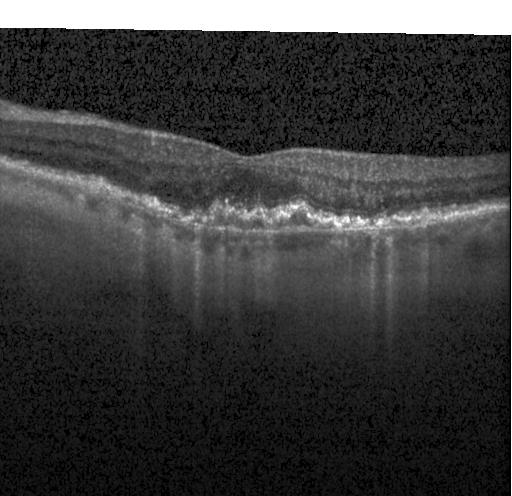
Retinal OCT cross-section — Dx: CNV.